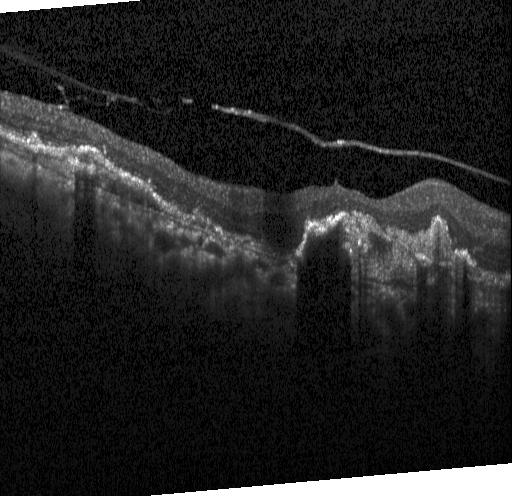
OCT B-scan showing choroidal neovascularization (CNV).